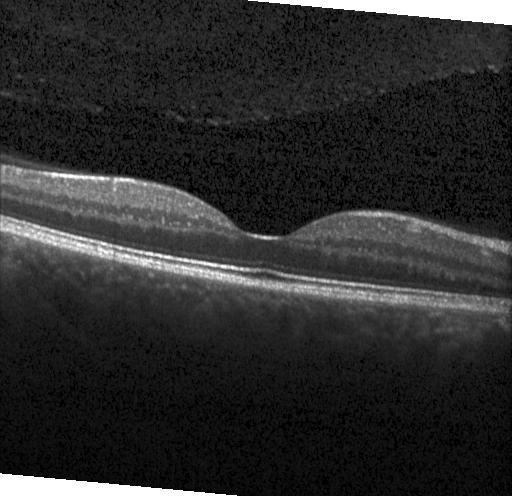 Heidelberg Spectralis OCT system. OCT line scan. Impression: neither choroidal neovascularization, diabetic macular edema, nor drusen.